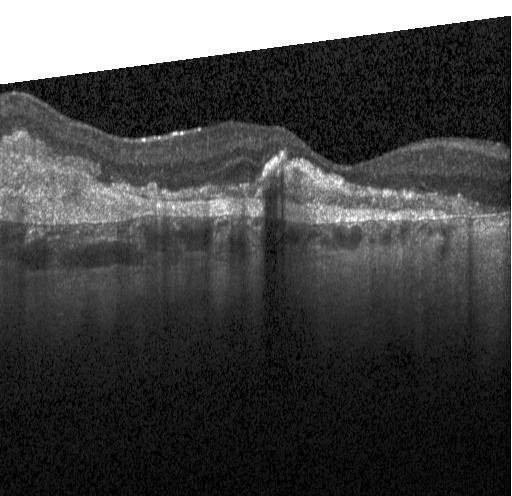 OCT B-scan showing choroidal neovascularization.